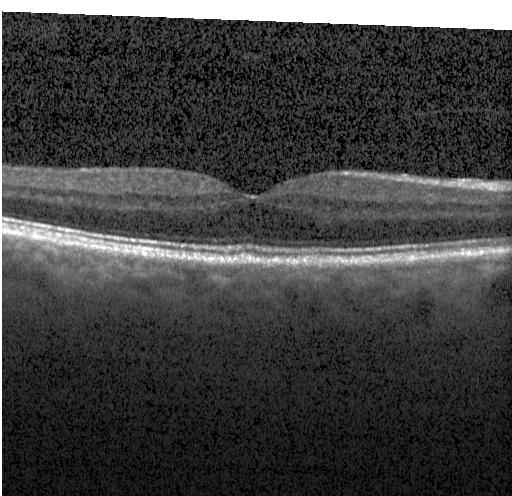

OCT B-scan. Finding: neither choroidal neovascularization, diabetic macular edema, nor drusen.